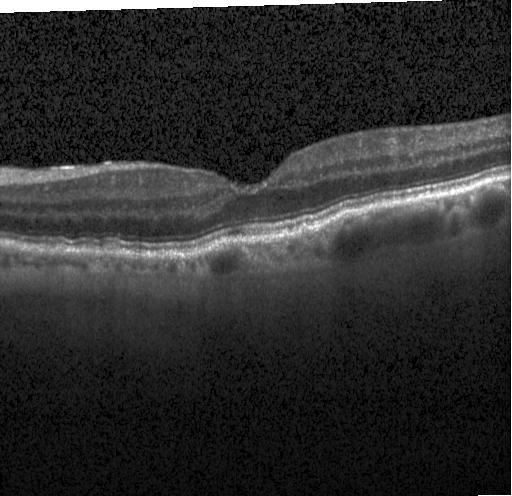

OCT finding: drusen.